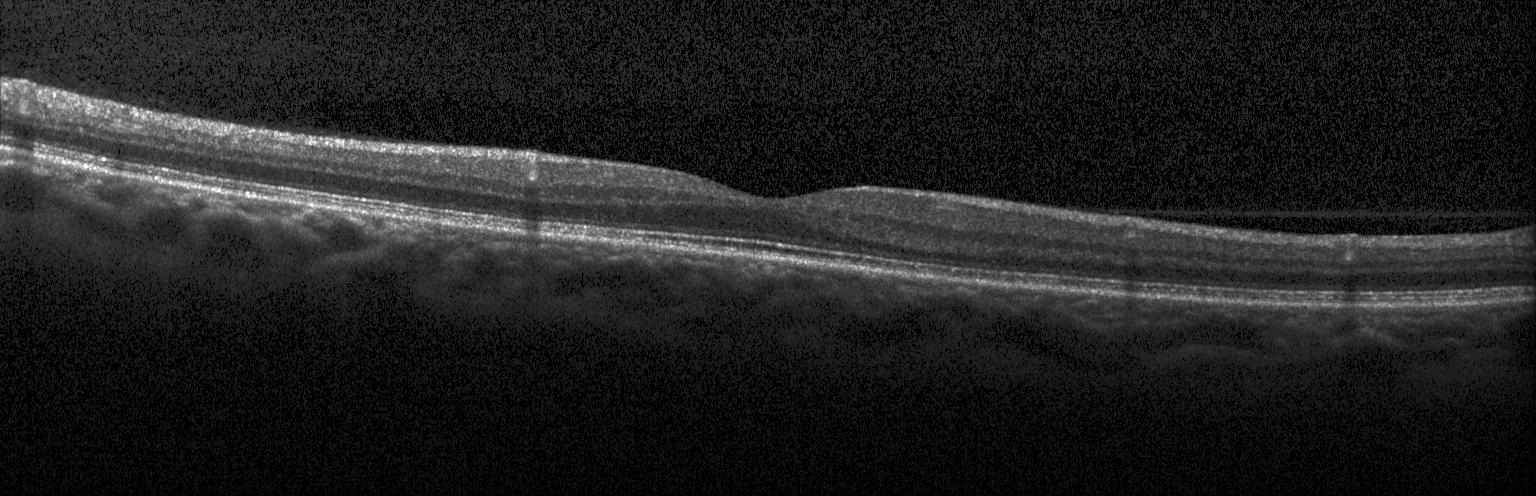 Acquired on a Heidelberg Spectralis · optical coherence tomography scan — Impression: no evidence of CNV, DME, or drusen.